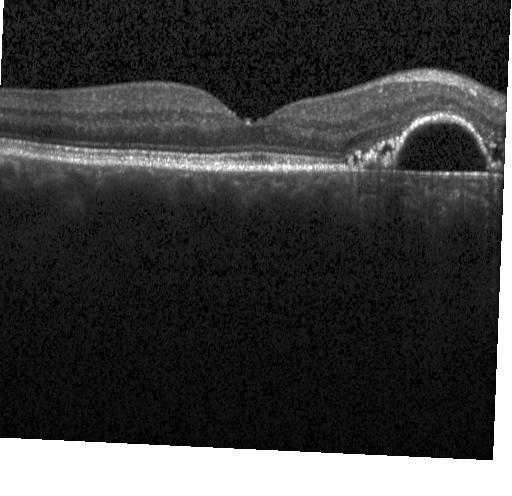

Optical coherence tomography scan; SD-OCT — A choroidal neovascular membrane.